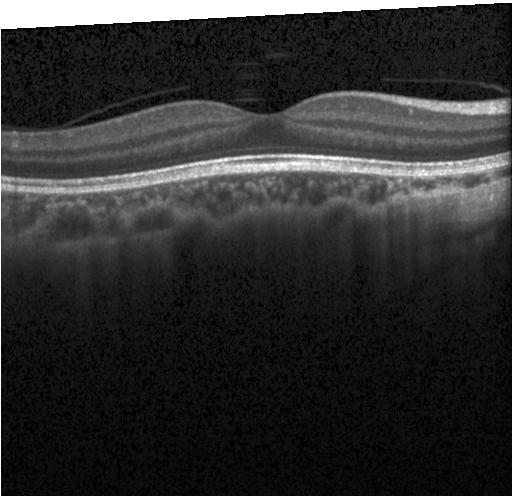

Instrument: Heidelberg Spectralis · optical coherence tomography B-scan — Finding: neither choroidal neovascularization, diabetic macular edema, nor drusen.